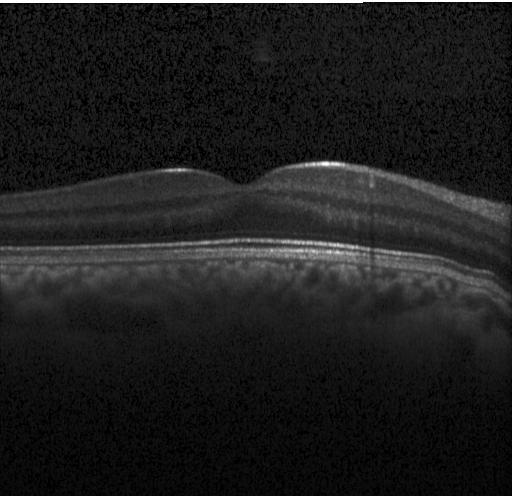 Finding: no evidence of choroidal neovascularization, diabetic macular edema, or drusen.